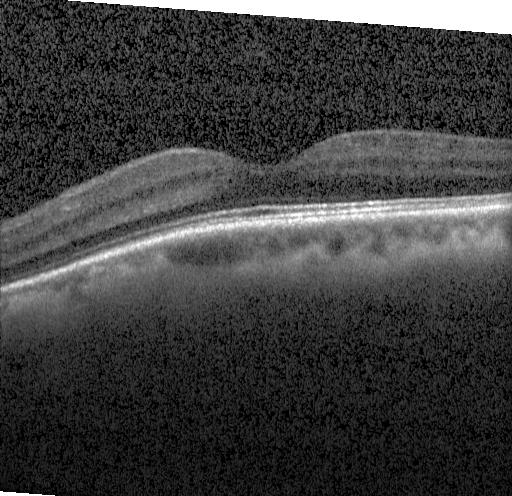

Retinal OCT cross-section showing no CNV, DME, or drusen.